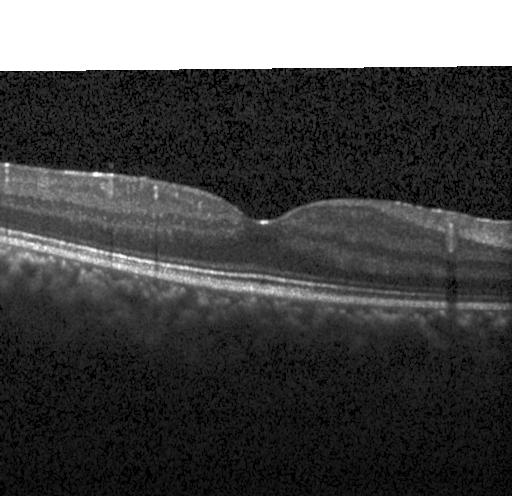

This B-scan demonstrates no evidence of choroidal neovascularization, diabetic macular edema, or drusen.